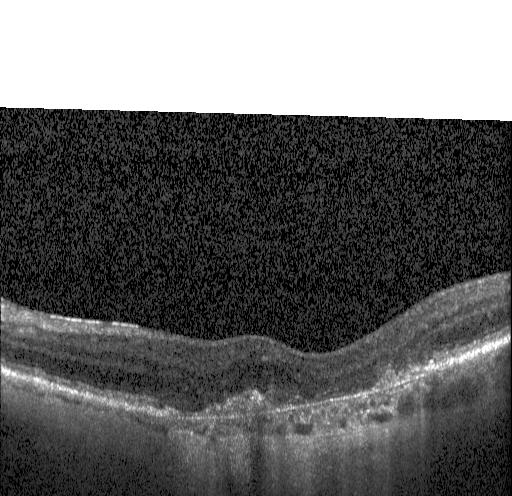

Retinal OCT B-scan · horizontal scan through the fovea · Heidelberg Spectralis OCT system. The scan shows a choroidal neovascular membrane.